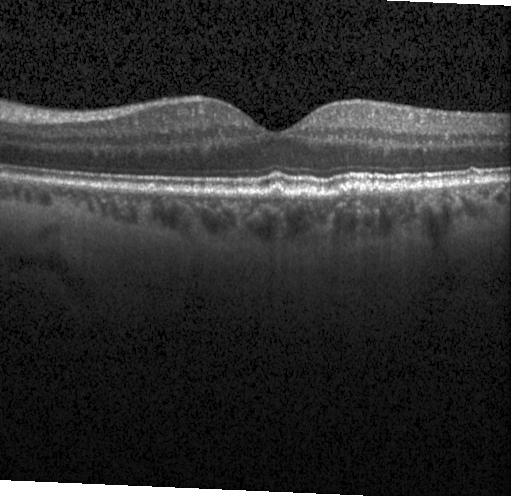
Diagnosis: drusen.